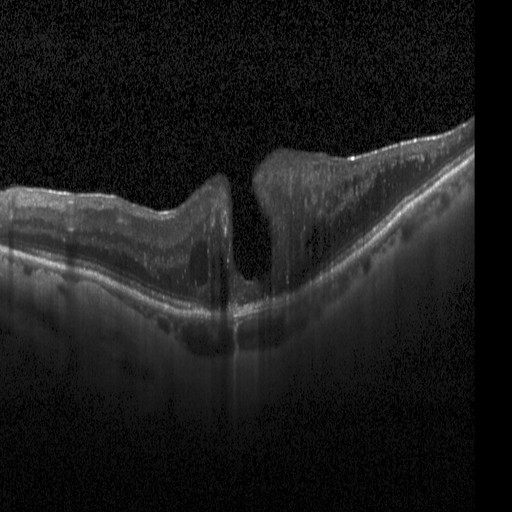

Retinal OCT cross-section
Assessment: diabetic macular edema.